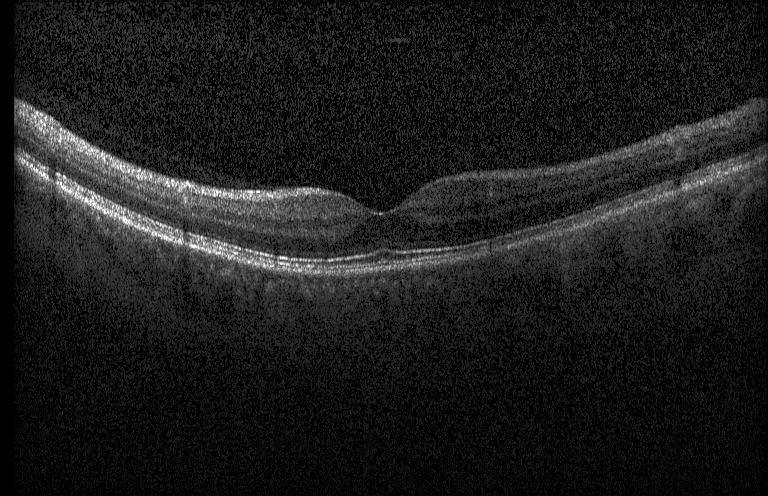 Horizontal scan through the fovea, retinal OCT cross-section — Impression: no choroidal neovascularization, diabetic macular edema, or drusen.